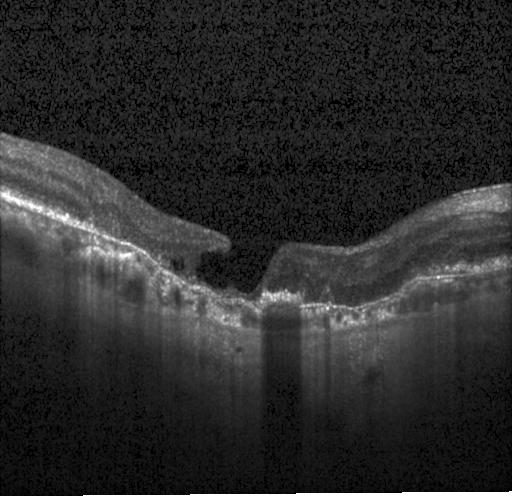

Spectral-domain OCT · through the macula · optical coherence tomography B-scan. Choroidal neovascularization (CNV).